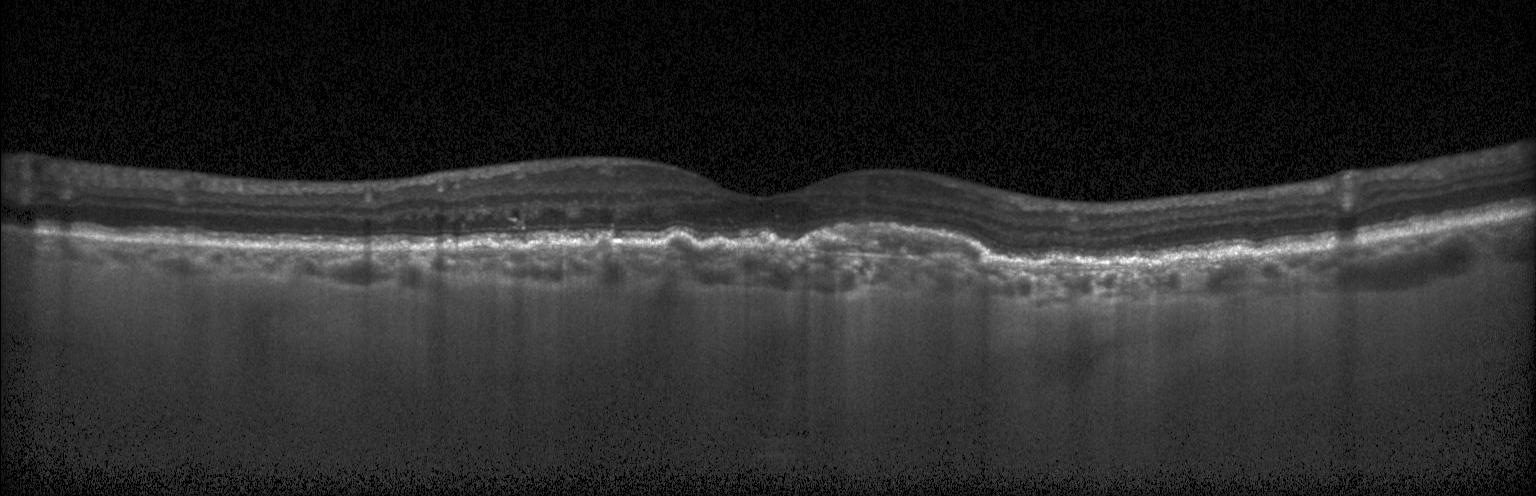 Optical coherence tomography B-scan — Macular OCT: choroidal neovascularization (CNV).